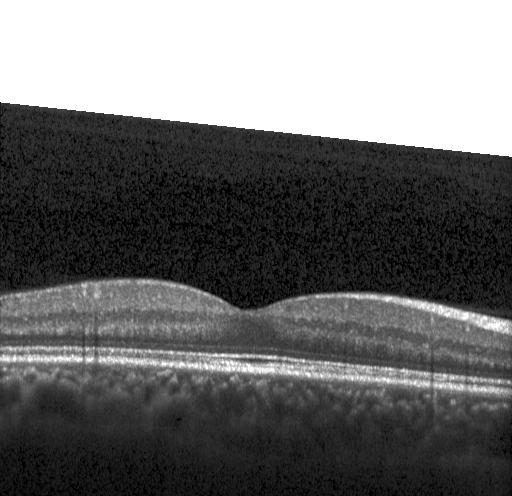
Spectral-domain optical coherence tomography; retinal OCT B-scan — This B-scan demonstrates neither choroidal neovascularization, diabetic macular edema, nor drusen.